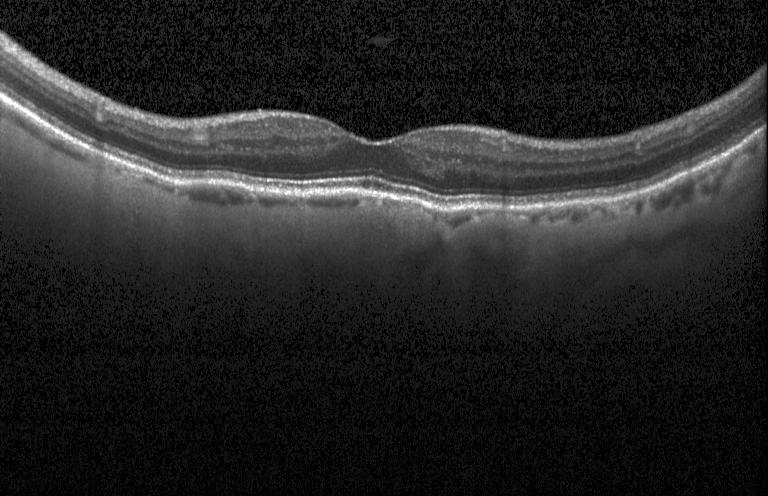

Diagnosis: no choroidal neovascularization, no diabetic macular edema, and no drusen.